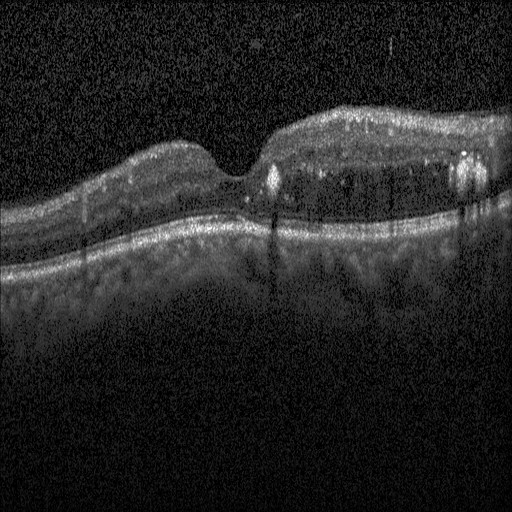
The scan shows diabetic macular edema (DME).